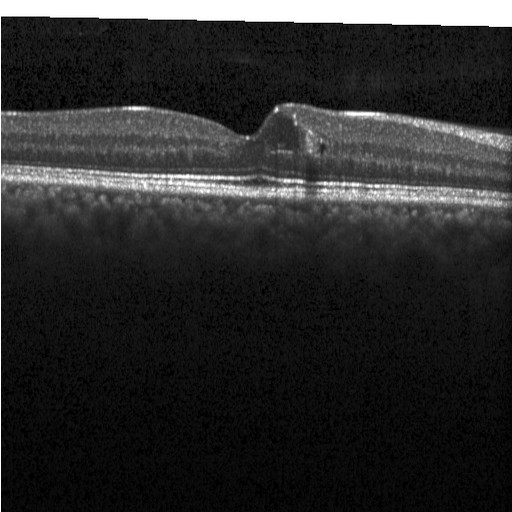 OCT finding: diabetic macular edema (DME).